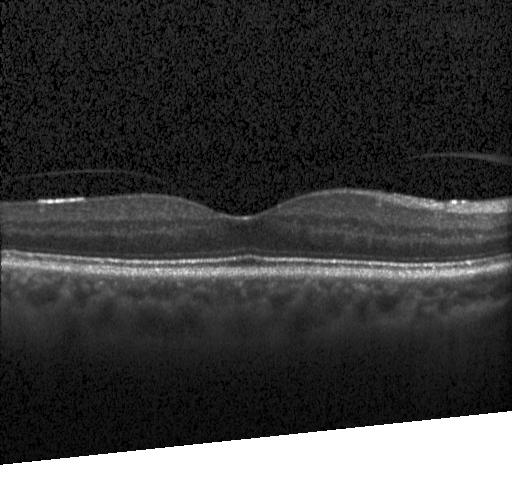
Finding: no CNV, no DME, and no drusen.